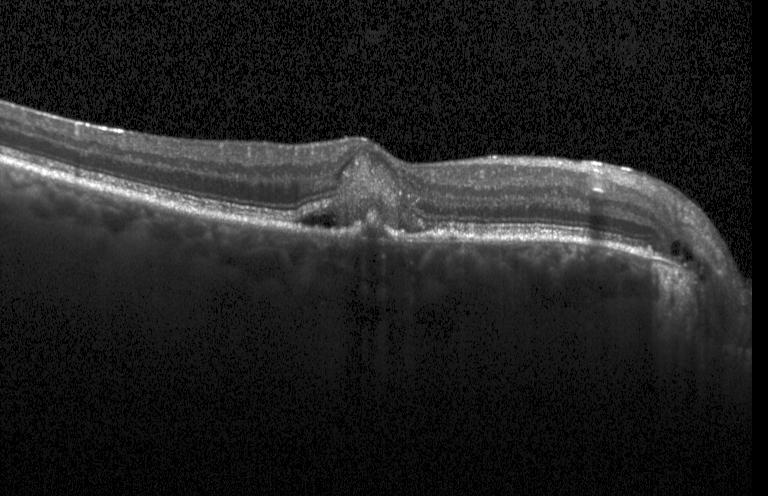
Optical coherence tomography scan; instrument: Heidelberg Spectralis; through the macula.
This B-scan demonstrates a choroidal neovascular membrane.